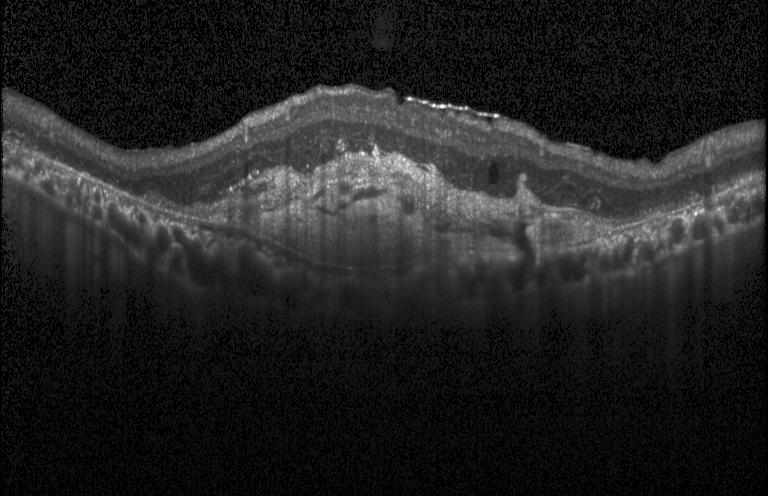
OCT B-scan. SD-OCT — Impression: a choroidal neovascular membrane.